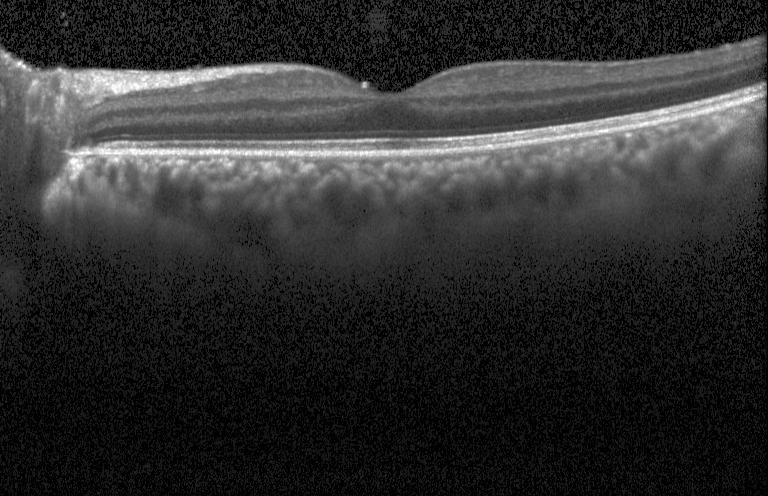
Retinal OCT cross-section. The scan shows no choroidal neovascularization, no diabetic macular edema, and no drusen.